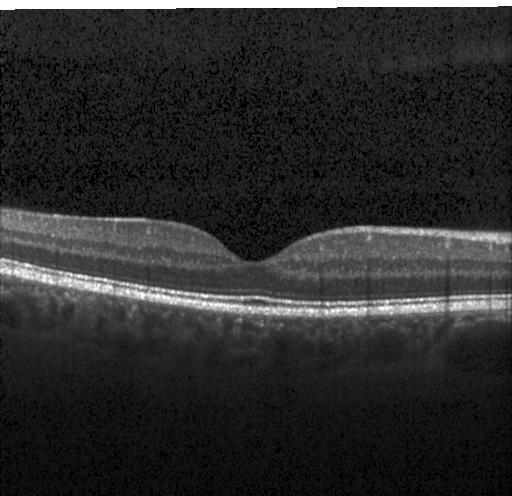 Diagnosis: no CNV, DME, or drusen.